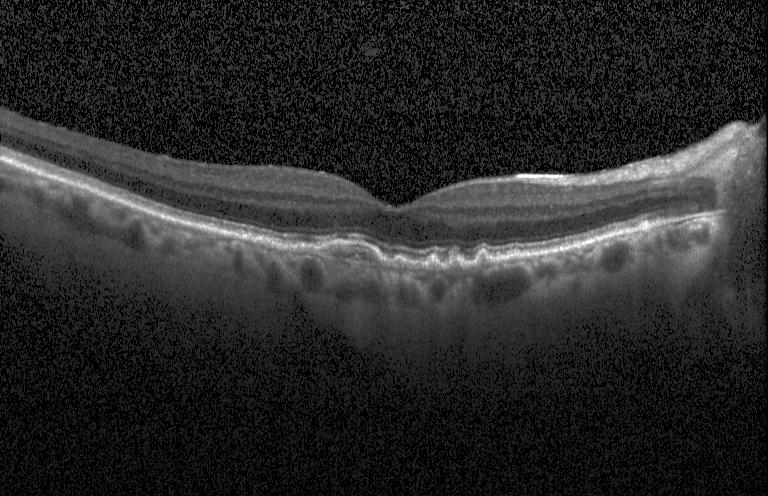
Spectral-domain optical coherence tomography. OCT B-scan. Acquired on a Heidelberg Spectralis. Centered on the fovea — Impression: choroidal neovascularization.